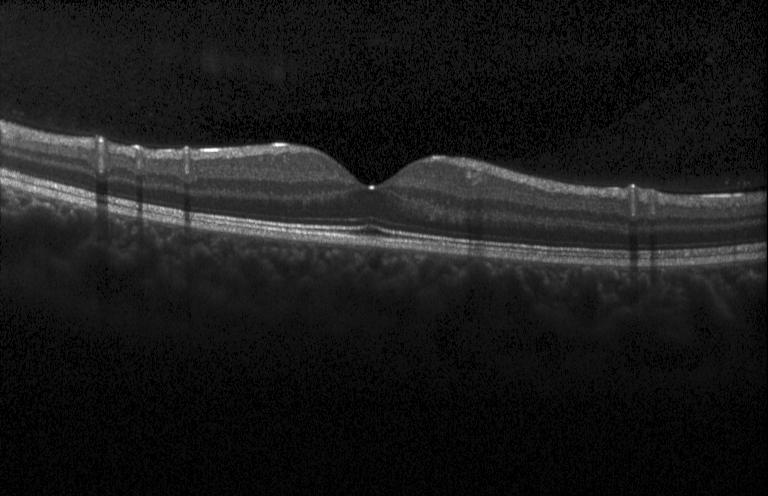
Retinal OCT cross-section · instrument: Heidelberg Spectralis · centered on the fovea — Dx: no choroidal neovascularization, diabetic macular edema, or drusen.